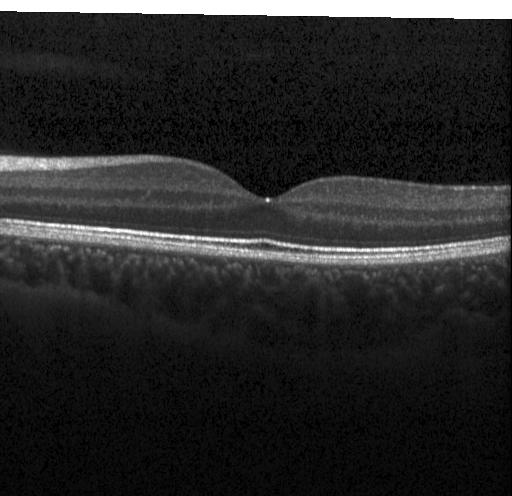

Spectral-domain OCT B-scan: no choroidal neovascularization, diabetic macular edema, or drusen.